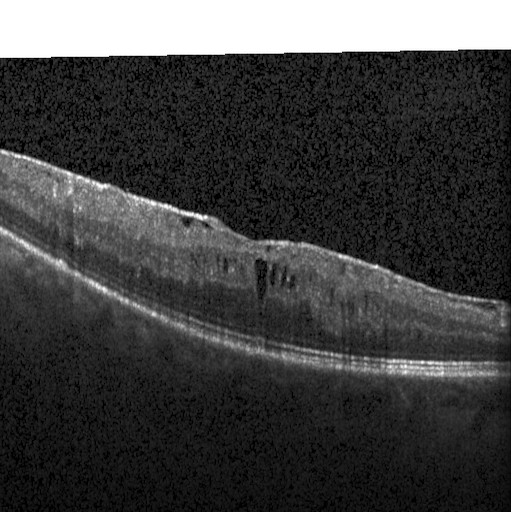 Macular scan · optical coherence tomography scan · acquired on a Heidelberg Spectralis
Finding: diabetic macular edema.